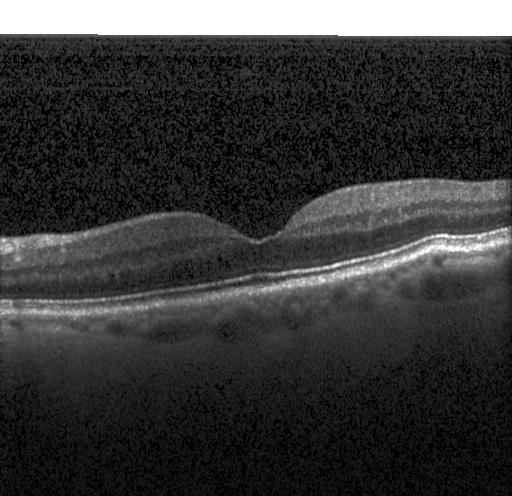
Optical coherence tomography scan. Finding: no CNV, no DME, and no drusen.